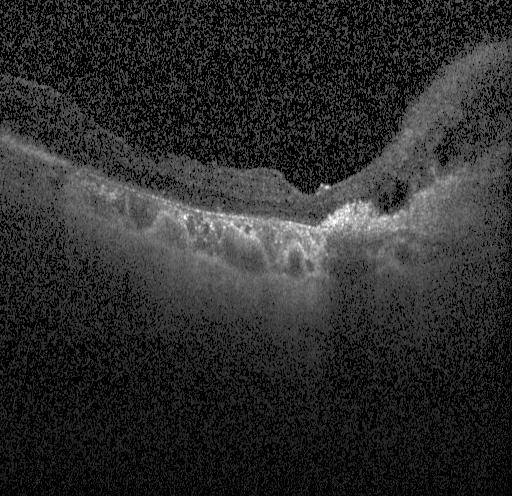
Spectral-domain OCT. Instrument: Heidelberg Spectralis. Through the macula. OCT B-scan — Diagnosis: a choroidal neovascular membrane.